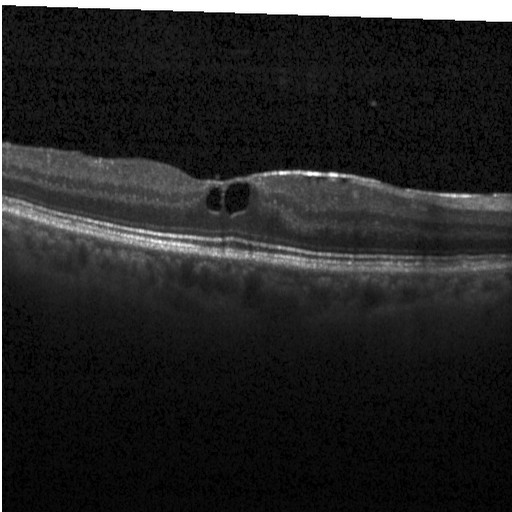

OCT scan showing DME.